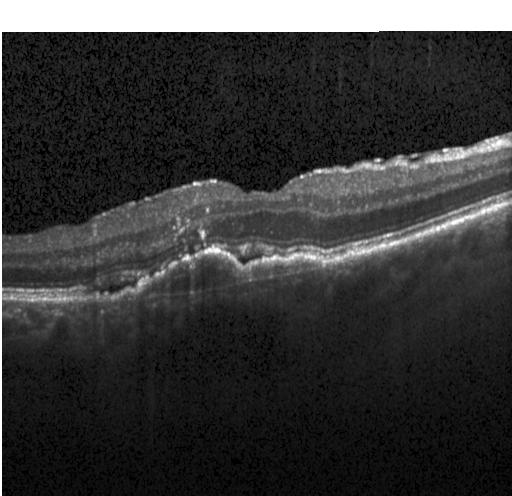 OCT line scan; spectral-domain OCT. Diagnosis: choroidal neovascularization (CNV).